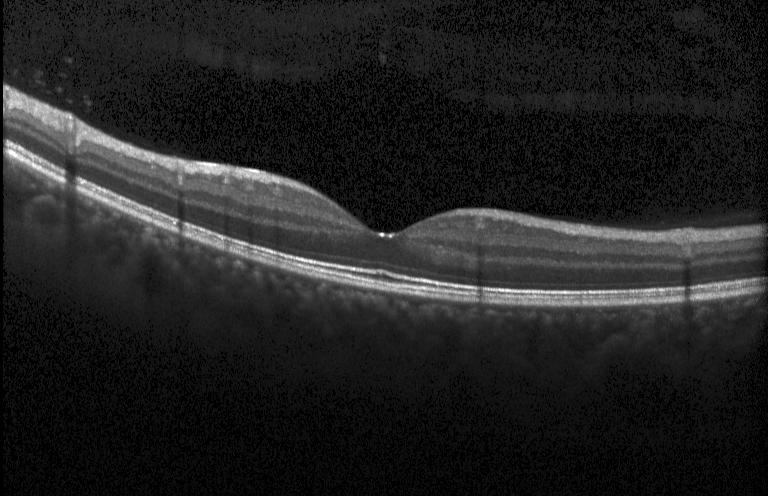

Finding: no choroidal neovascularization, diabetic macular edema, or drusen.